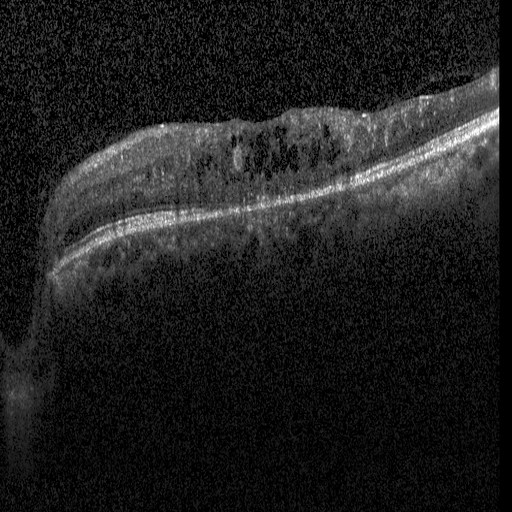
Fovea-centered. Retinal OCT cross-section — This B-scan demonstrates DME.